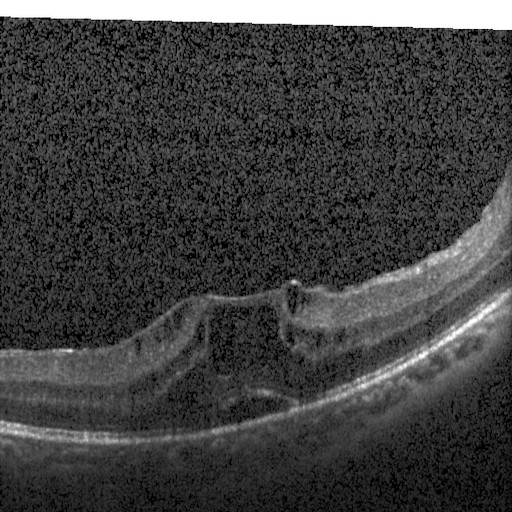 Impression: DME.